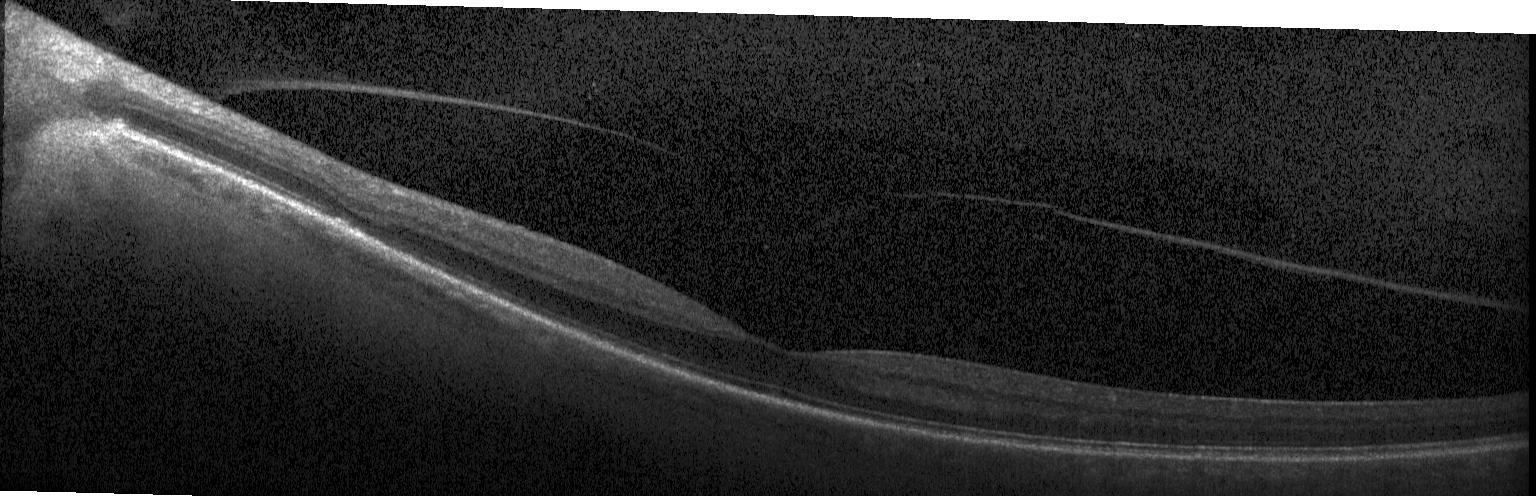
Spectral-domain optical coherence tomography, optical coherence tomography scan.
Diagnosis: no evidence of choroidal neovascularization, diabetic macular edema, or drusen.